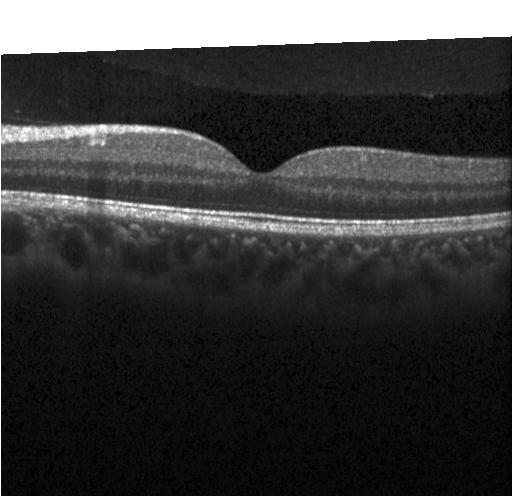 OCT B-scan, instrument: Heidelberg Spectralis, spectral-domain OCT — OCT finding: no evidence of CNV, DME, or drusen.